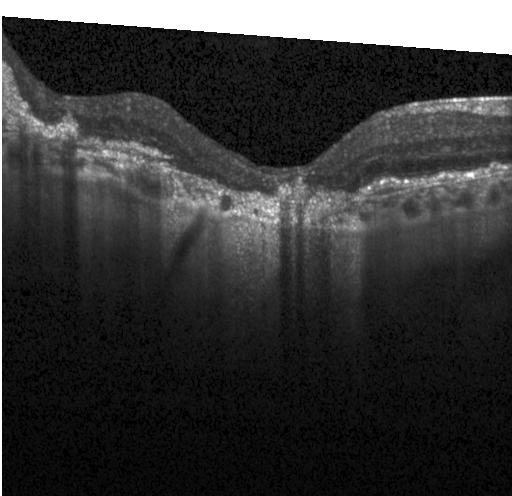

Retinal OCT B-scan, fovea-centered
Finding: a choroidal neovascular membrane.